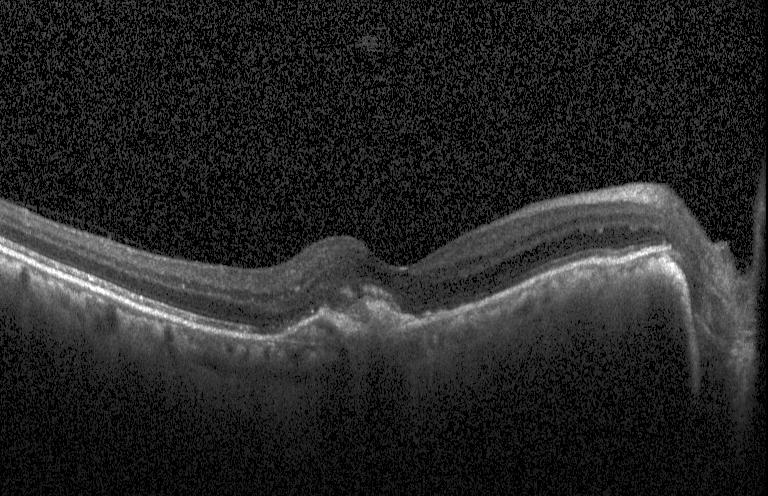

Diagnosis: a choroidal neovascular membrane.